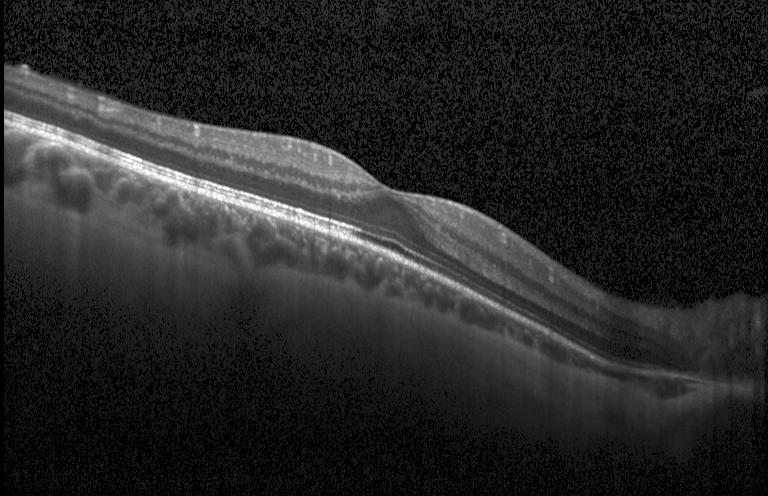
This B-scan demonstrates no choroidal neovascularization, no diabetic macular edema, and no drusen.